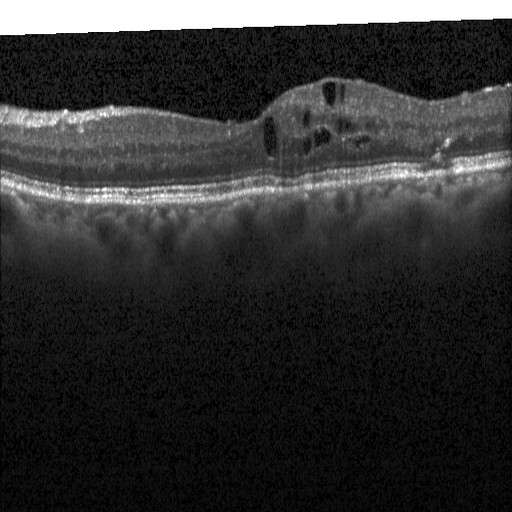 Spectral-domain optical coherence tomography. OCT line scan. Fovea-centered
Finding: diabetic macular edema.